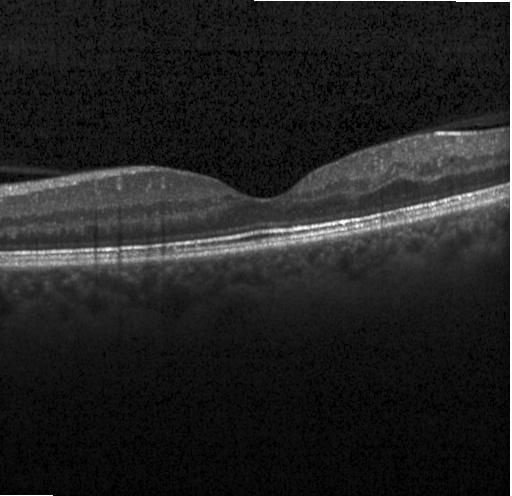

Fovea-centered · acquired on a Heidelberg Spectralis · OCT line scan · SD-OCT — Macular OCT: neither choroidal neovascularization, diabetic macular edema, nor drusen.